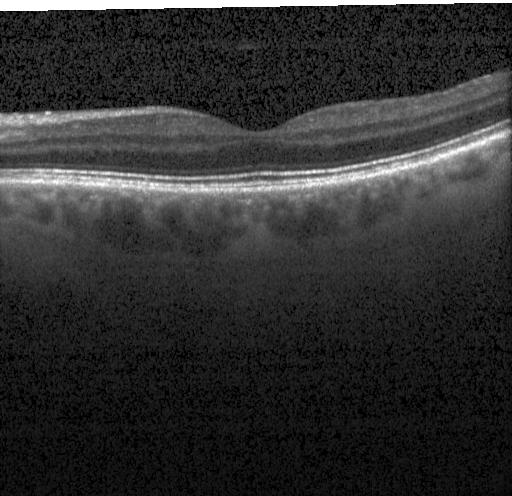

No choroidal neovascularization, no diabetic macular edema, and no drusen.